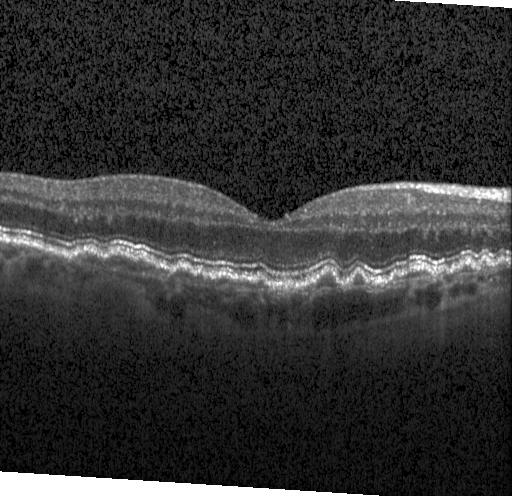
Spectral-domain OCT, retinal OCT cross-section, horizontal scan through the fovea, instrument: Heidelberg Spectralis — Impression: multiple drusen.